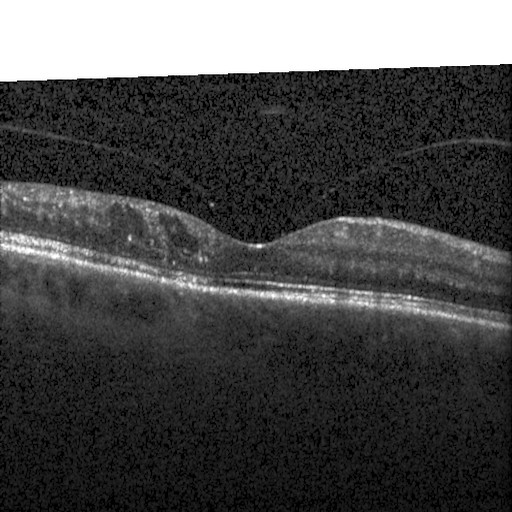 Optical coherence tomography scan
Diagnosis: DME.